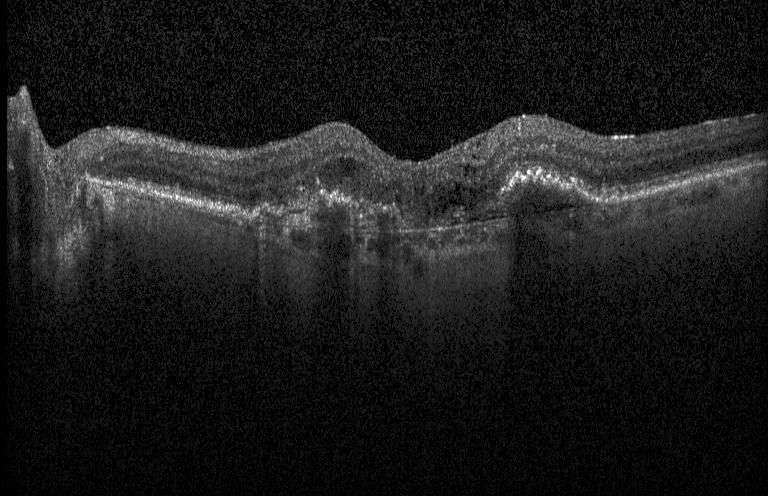 OCT line scan. Centered on the fovea. Acquired on a Heidelberg Spectralis
CNV.